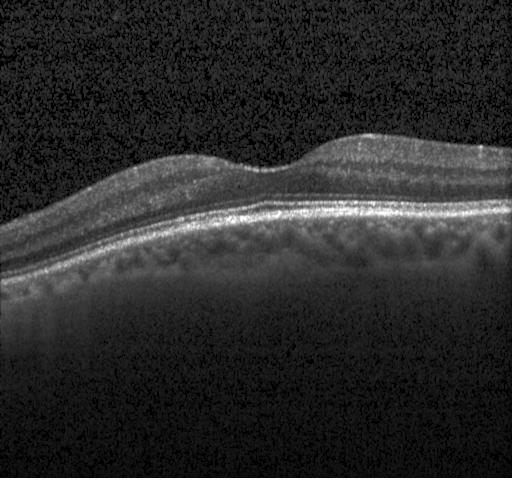
Optical coherence tomography scan.
Diagnosis: no evidence of CNV, DME, or drusen.